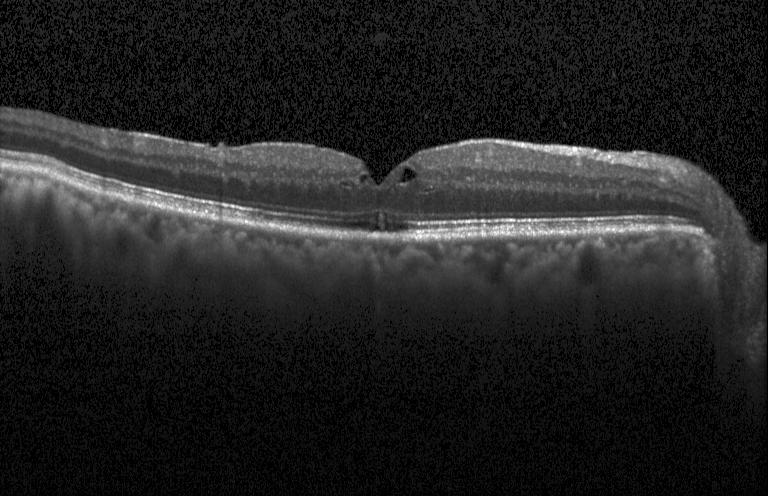

Spectral-domain optical coherence tomography · retinal OCT B-scan · instrument: Heidelberg Spectralis · horizontal scan through the fovea — Impression: diabetic macular edema (DME).